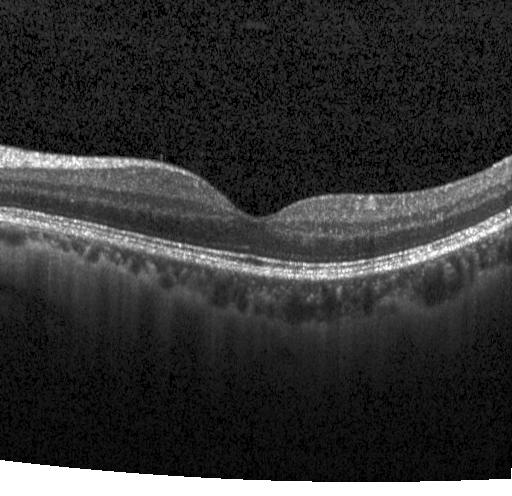

Retinal OCT cross-section showing no evidence of CNV, DME, or drusen.